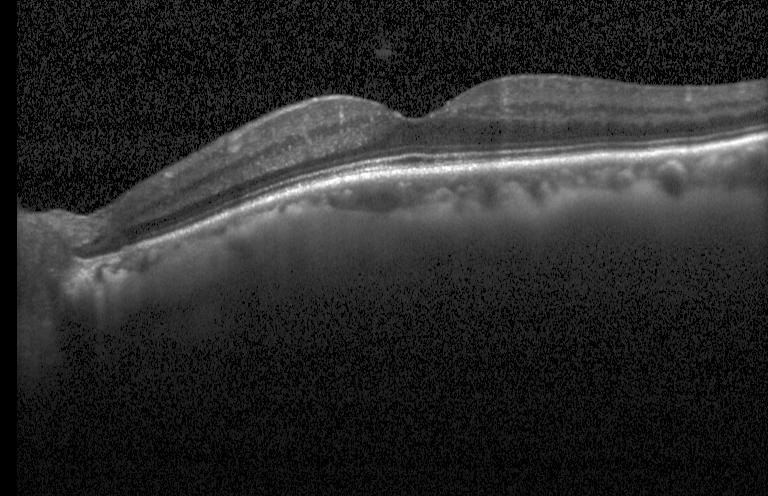
Impression: no CNV, no DME, and no drusen.